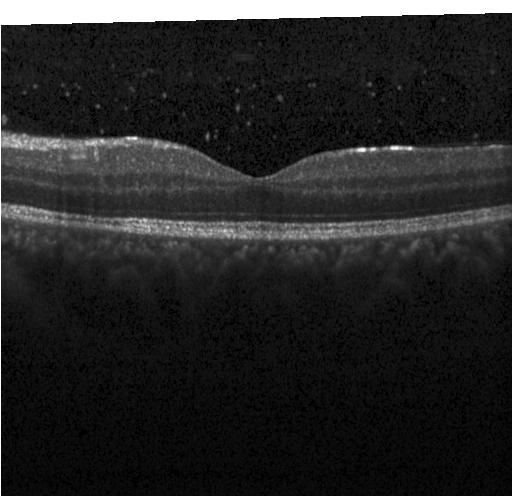 Neither CNV, DME, nor drusen.